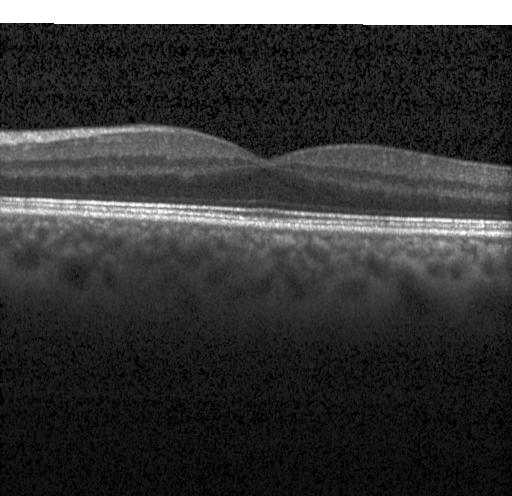

Impression: neither choroidal neovascularization, diabetic macular edema, nor drusen.